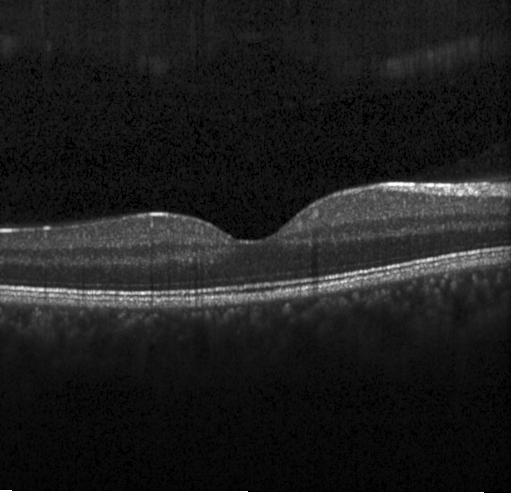
Centered on the fovea · optical coherence tomography B-scan · Heidelberg Spectralis OCT system
Diagnosis: no CNV, DME, or drusen.